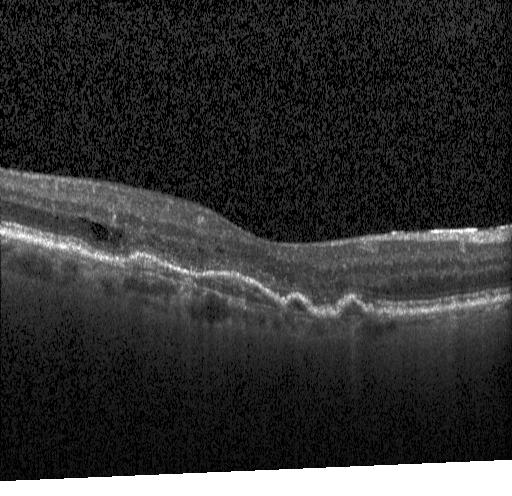 Finding: choroidal neovascularization.